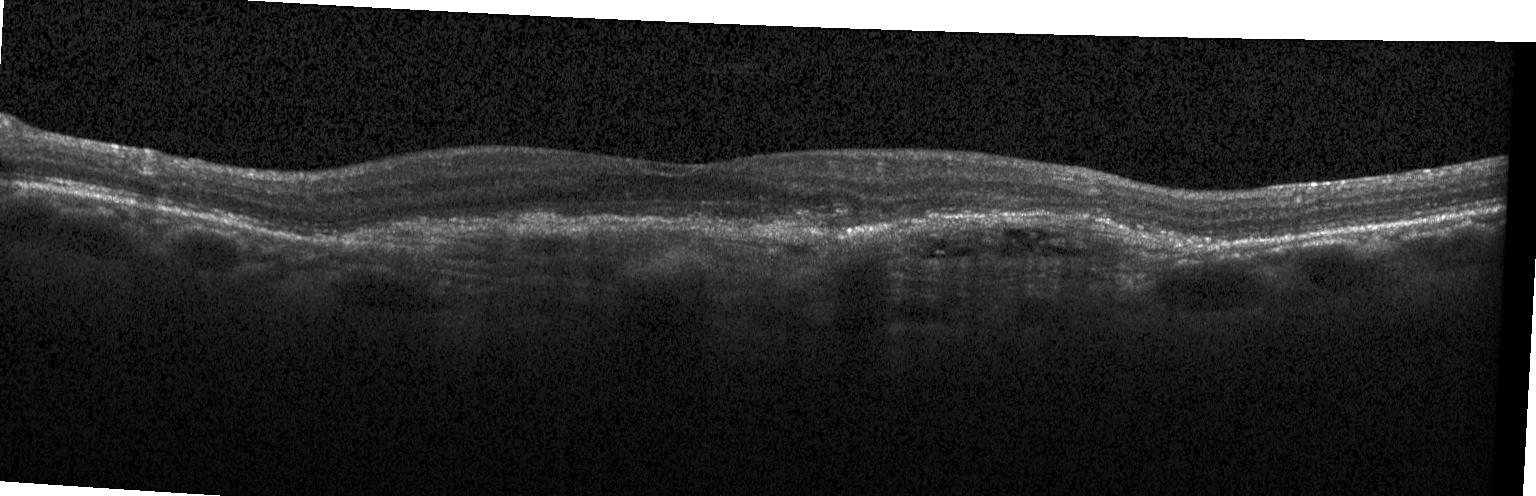
OCT finding: a choroidal neovascular membrane.